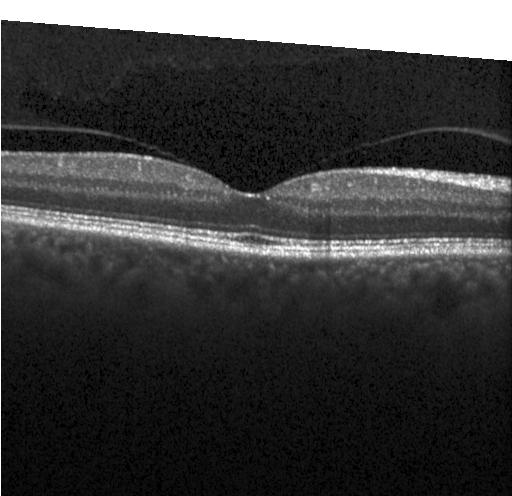 Impression: no choroidal neovascularization, no diabetic macular edema, and no drusen.